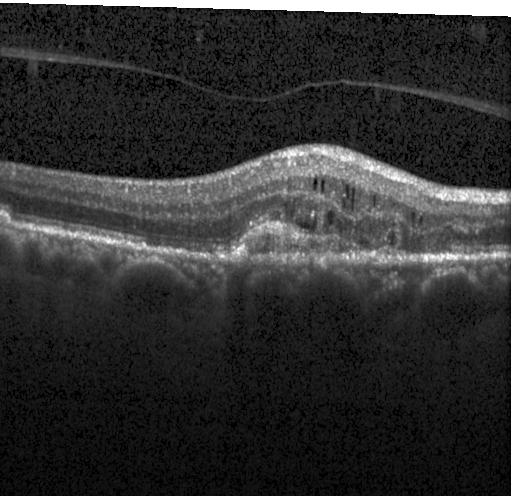
Spectral-domain OCT · optical coherence tomography B-scan · Heidelberg Spectralis OCT system
Impression: a choroidal neovascular membrane.